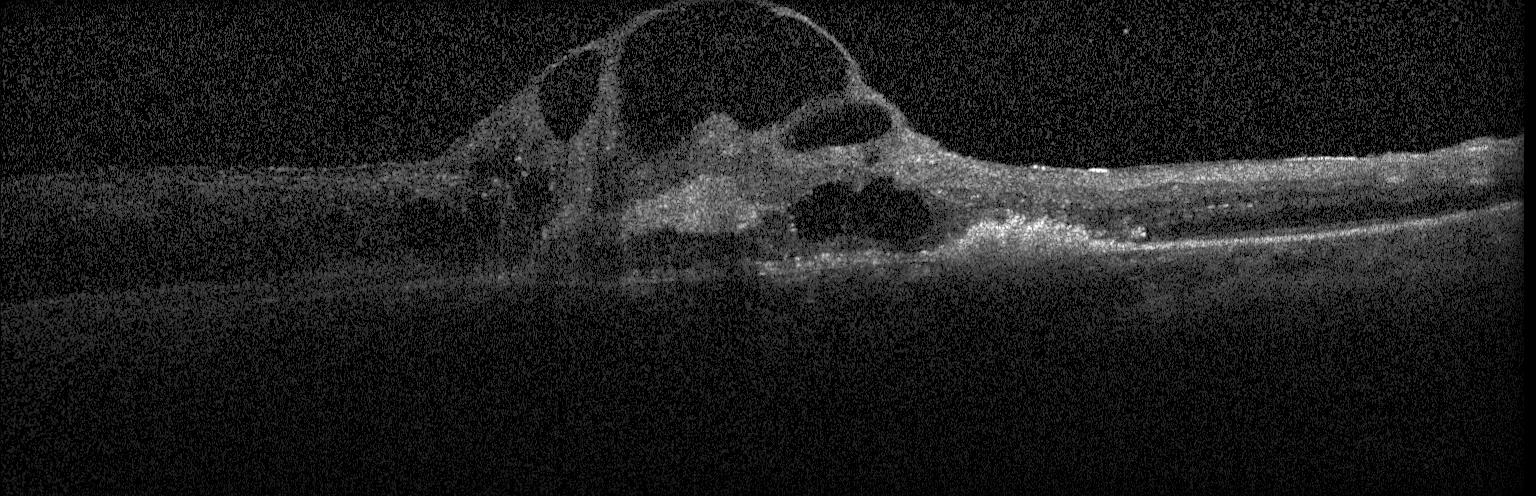

OCT scan showing CNV.